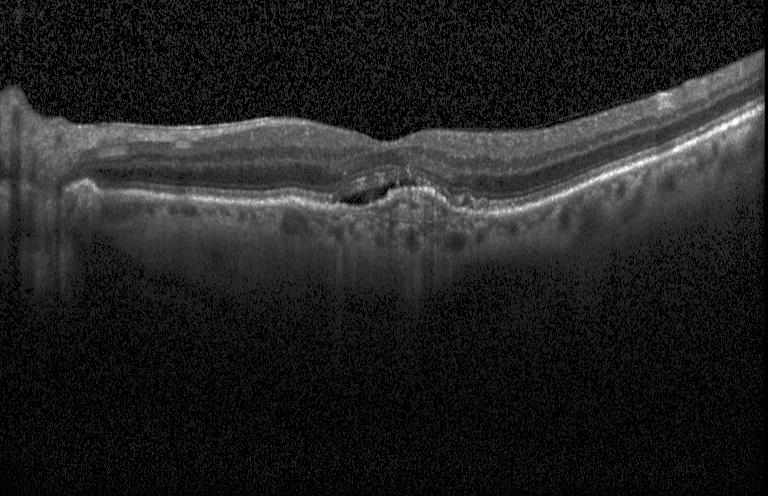
Spectral-domain optical coherence tomography; optical coherence tomography scan; fovea-centered.
Impression: a choroidal neovascular membrane.